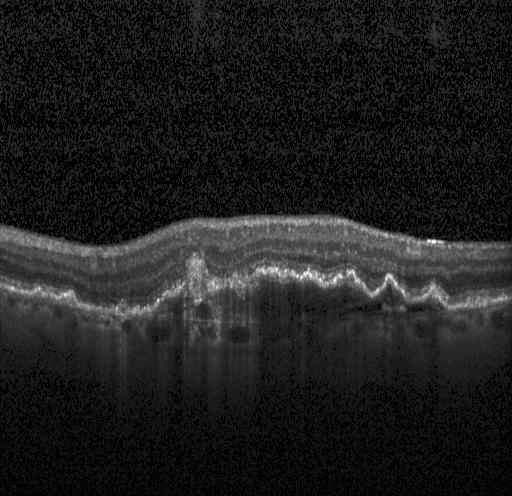

Finding: choroidal neovascularization (CNV).